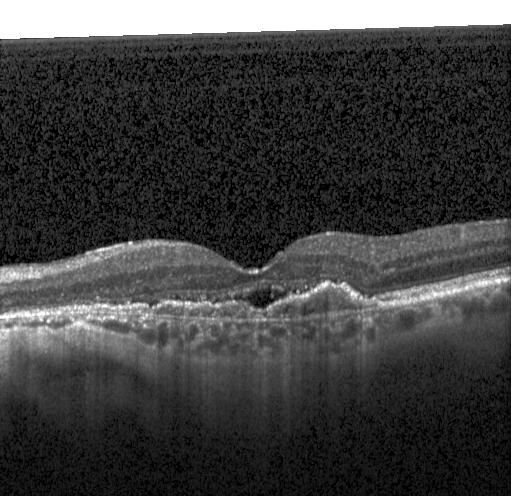
This B-scan demonstrates choroidal neovascularization.